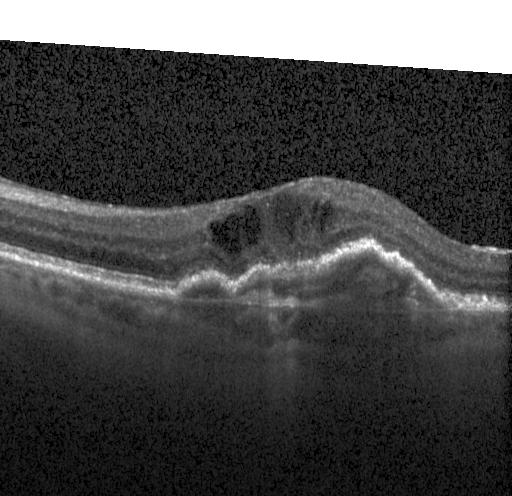 Diagnosis: a choroidal neovascular membrane.